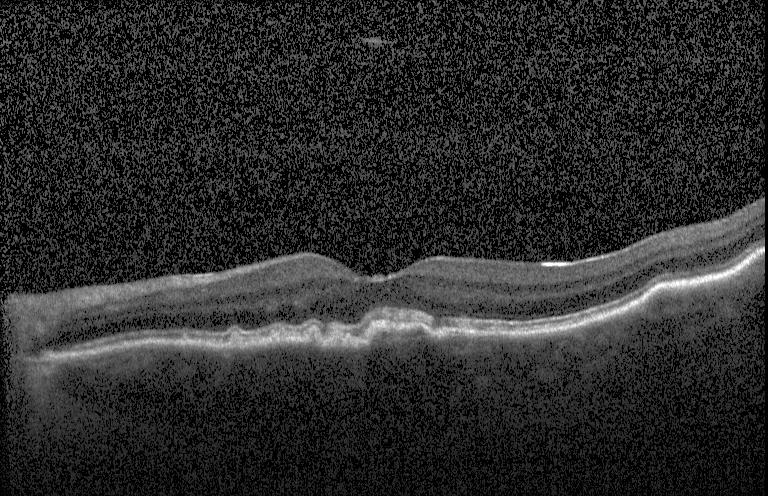
OCT B-scan showing drusen.